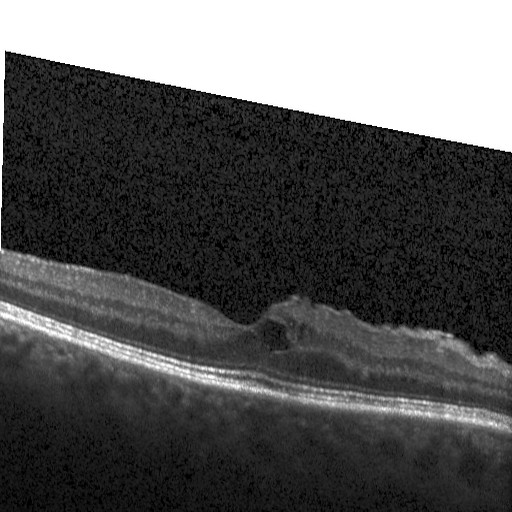

Spectral-domain optical coherence tomography. OCT B-scan — This B-scan demonstrates DME.